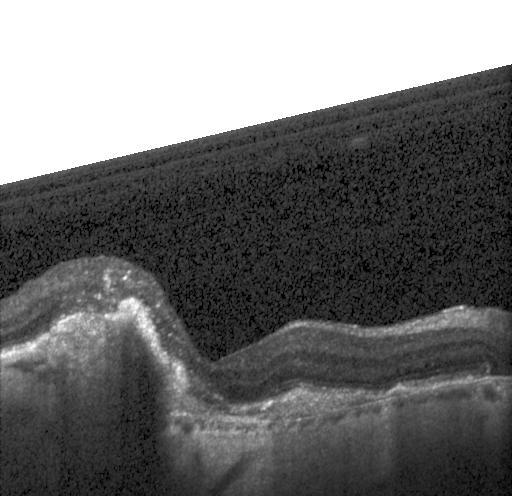 Acquired on a Heidelberg Spectralis. Retinal OCT B-scan. This B-scan demonstrates a choroidal neovascular membrane.